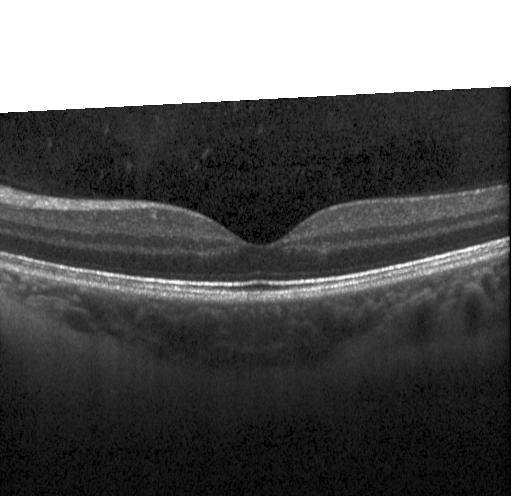

Optical coherence tomography B-scan · instrument: Heidelberg Spectralis.
Impression: no choroidal neovascularization, no diabetic macular edema, and no drusen.